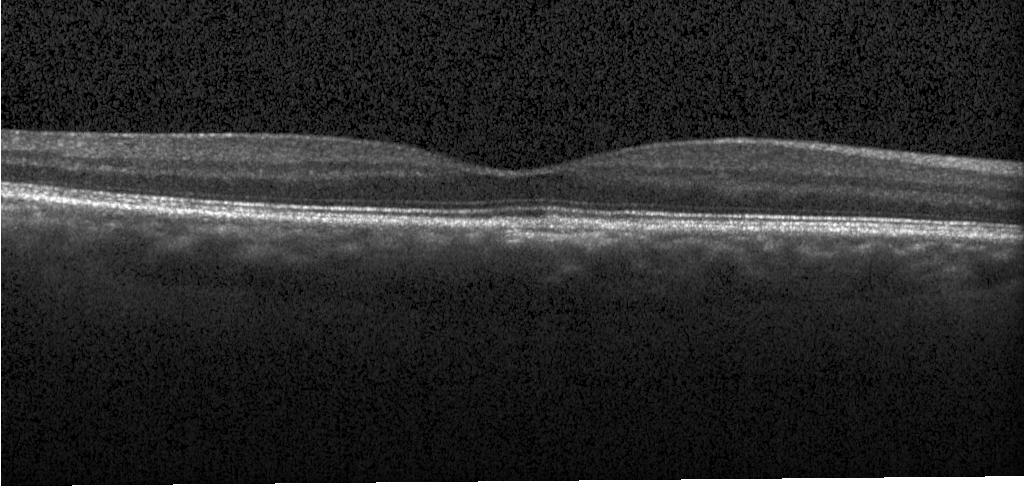
Macular OCT: neither choroidal neovascularization, diabetic macular edema, nor drusen.